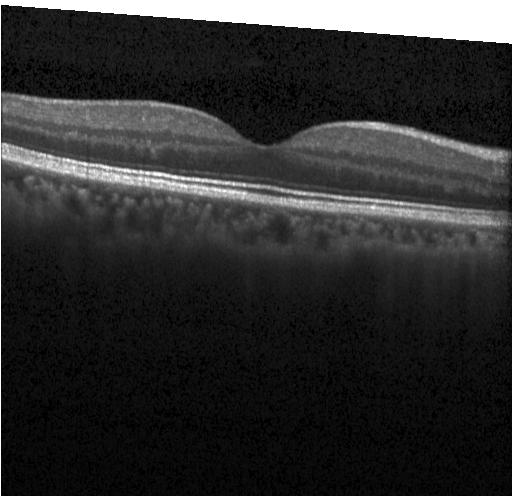

Retinal OCT cross-section. Instrument: Heidelberg Spectralis. Spectral-domain optical coherence tomography — OCT finding: no CNV, DME, or drusen.